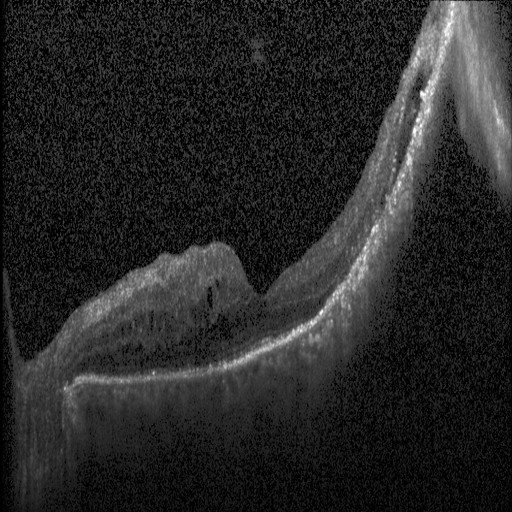
Macular scan. Optical coherence tomography scan
Diagnosis: diabetic macular edema (DME).